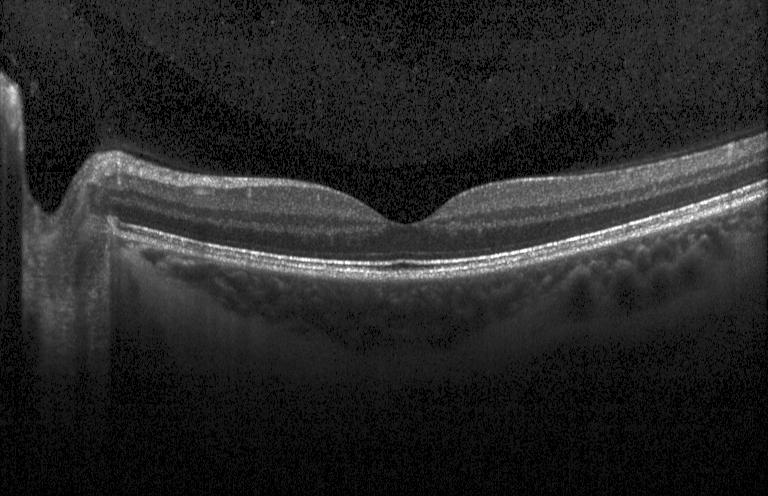
Heidelberg Spectralis · retinal OCT B-scan · through the macula.
Impression: no evidence of CNV, DME, or drusen.